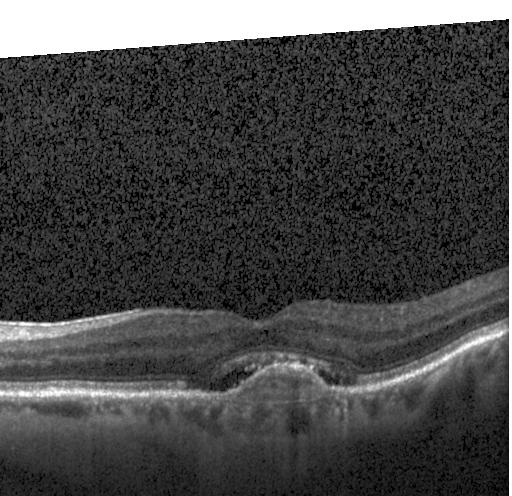

Retinal OCT B-scan — Assessment: a choroidal neovascular membrane.